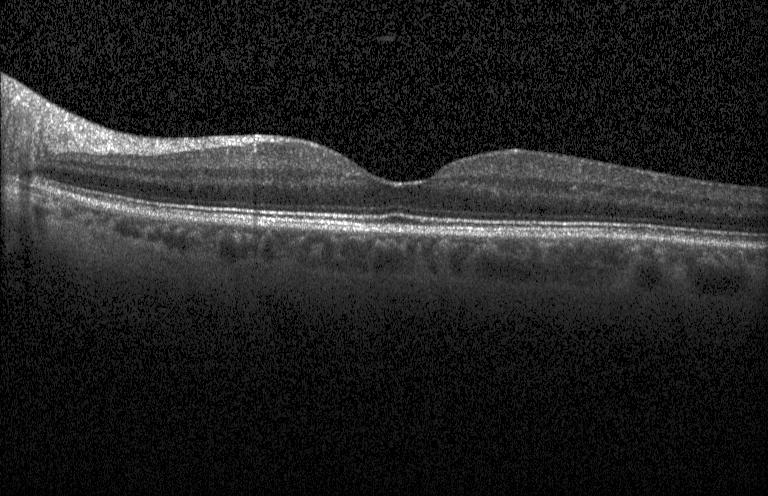

Macular OCT demonstrating no evidence of choroidal neovascularization, diabetic macular edema, or drusen.